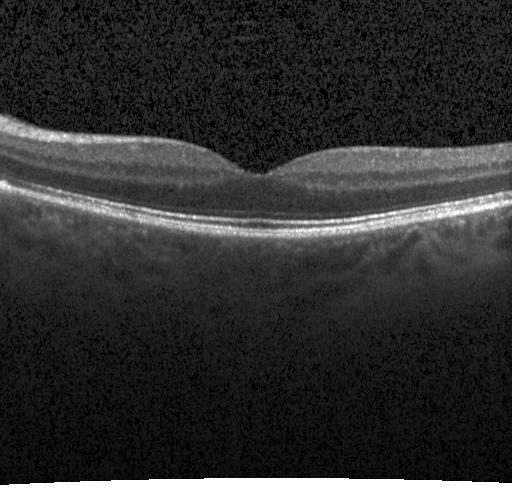 SD-OCT; optical coherence tomography scan.
Diagnosis: no evidence of CNV, DME, or drusen.